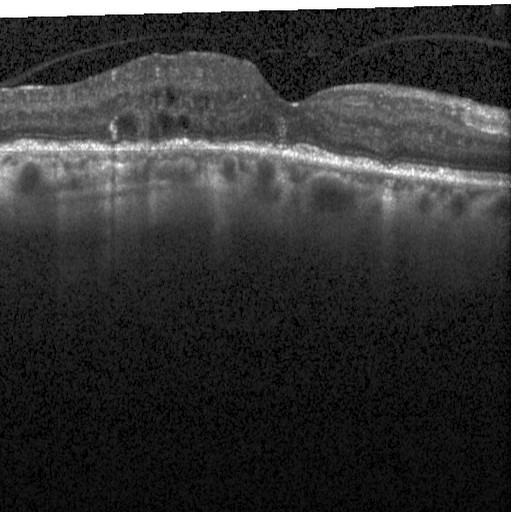
OCT line scan — Diagnosis: diabetic macular edema.